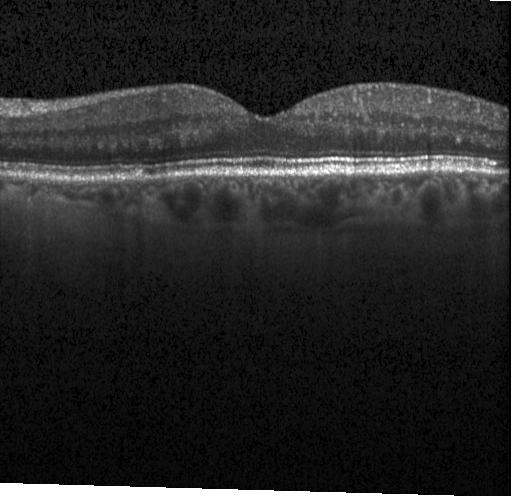 Instrument: Heidelberg Spectralis; spectral-domain optical coherence tomography; OCT line scan; macular scan
Diagnosis: no evidence of choroidal neovascularization, diabetic macular edema, or drusen.